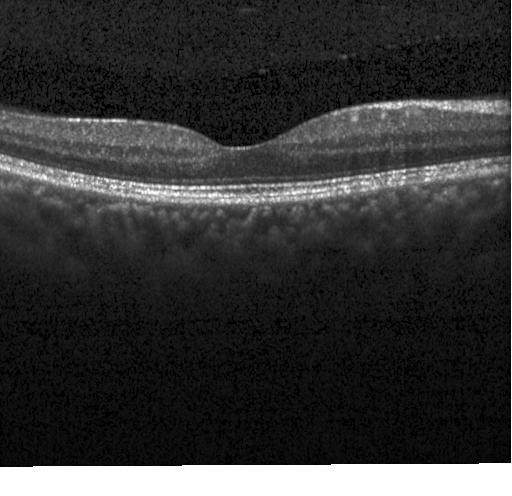
Assessment: no CNV, DME, or drusen.